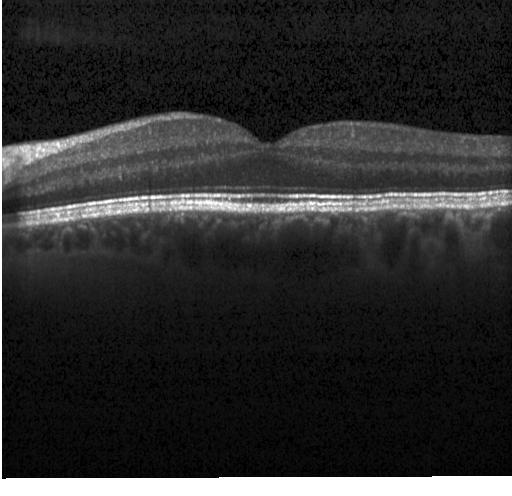 Diagnosis: no choroidal neovascularization, diabetic macular edema, or drusen.